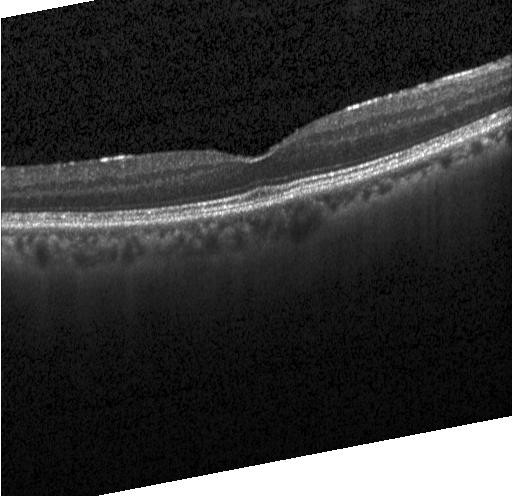

Diagnosis: no evidence of choroidal neovascularization, diabetic macular edema, or drusen.